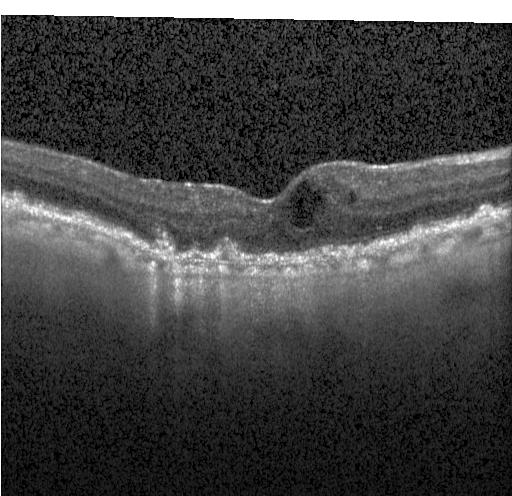
Finding: choroidal neovascularization (CNV).